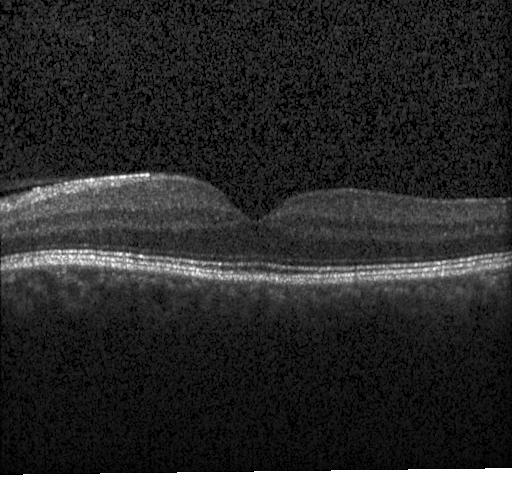
OCT B-scan.
Finding: no choroidal neovascularization, no diabetic macular edema, and no drusen.